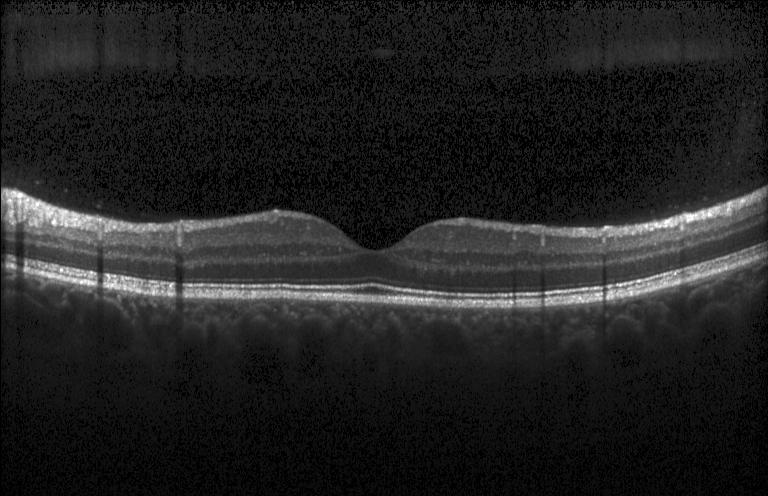

Finding: no CNV, DME, or drusen.